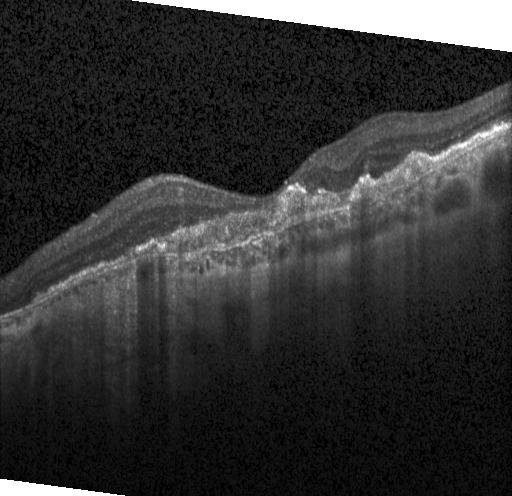 Acquired on a Heidelberg Spectralis; SD-OCT; horizontal scan through the fovea; OCT B-scan. Diagnosis: choroidal neovascularization (CNV).